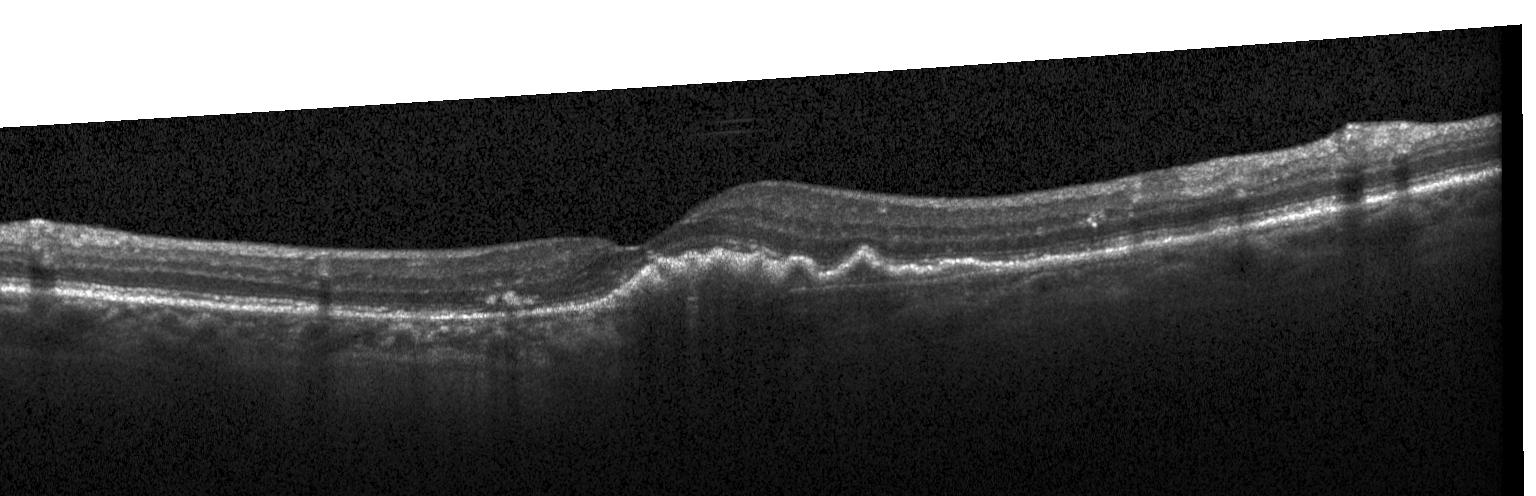

OCT line scan, centered on the fovea.
Impression: choroidal neovascularization.